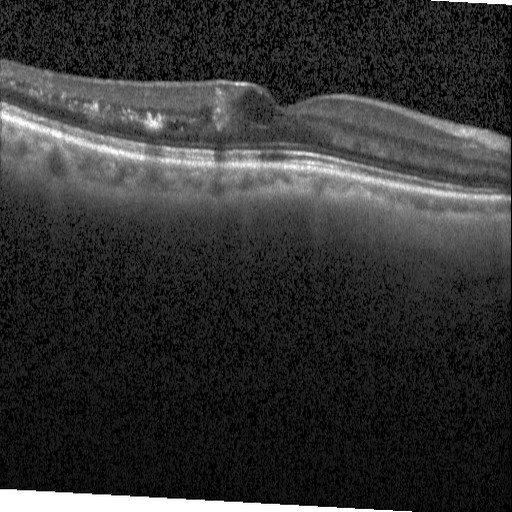
OCT line scan. Diagnosis: diabetic macular edema.